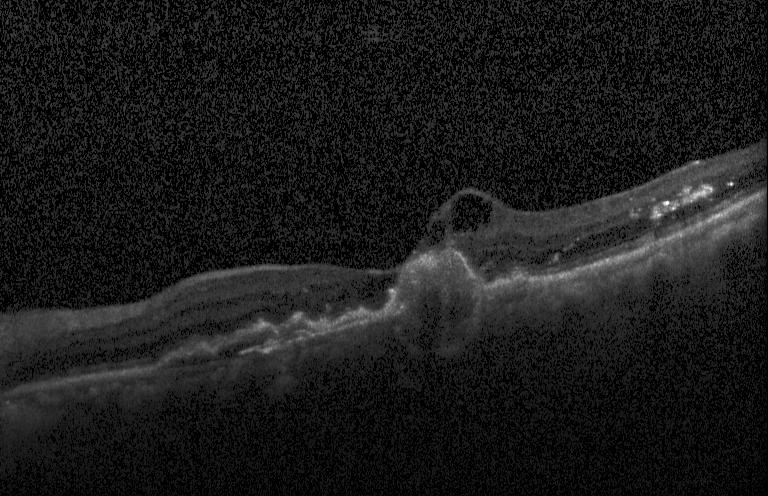

OCT scan showing a choroidal neovascular membrane.